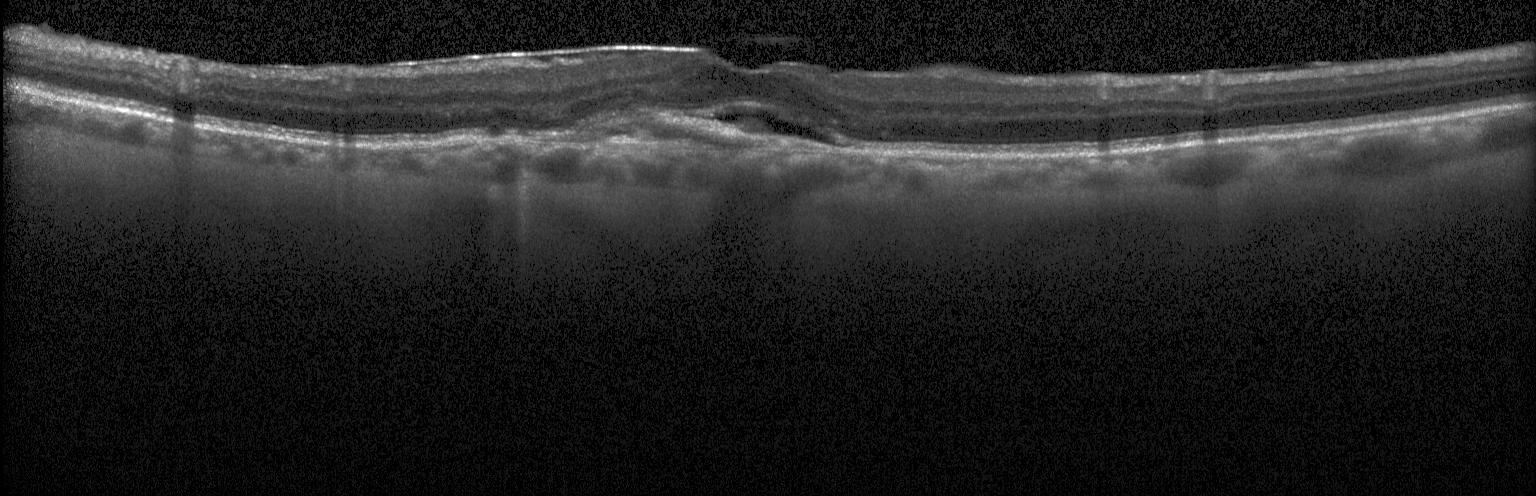
This B-scan demonstrates choroidal neovascularization.